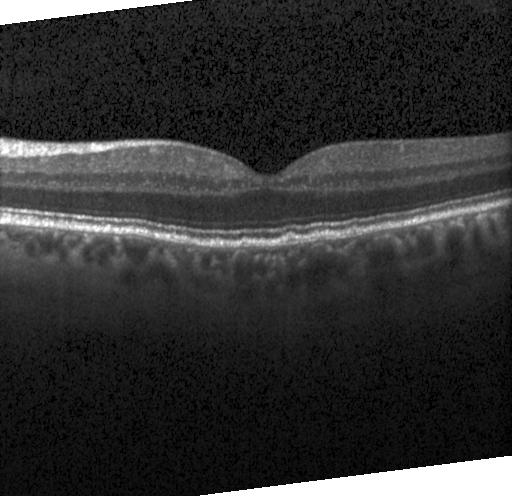 Optical coherence tomography B-scan, fovea-centered.
Impression: multiple drusen.